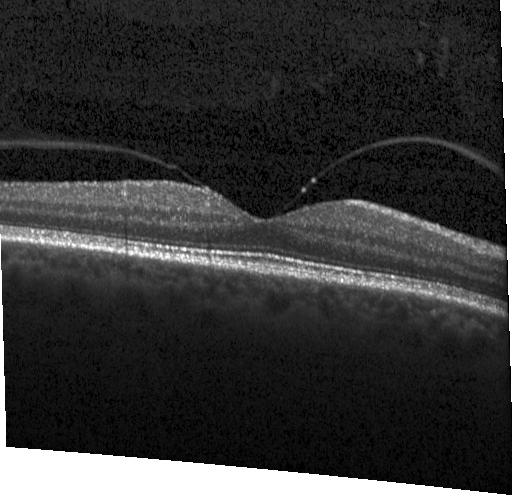
Heidelberg Spectralis OCT system. Fovea-centered. OCT line scan.
Diagnosis: no CNV, no DME, and no drusen.